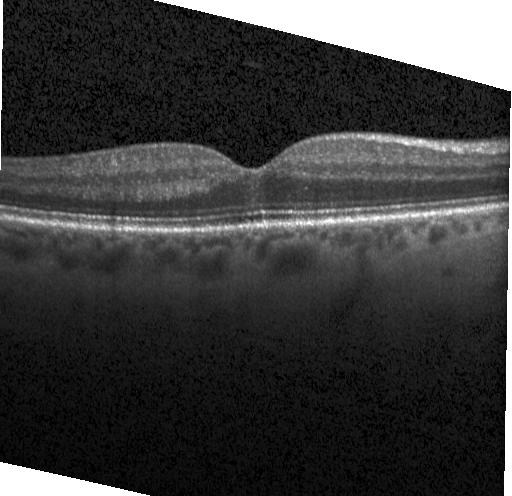

Macular OCT: neither CNV, DME, nor drusen.